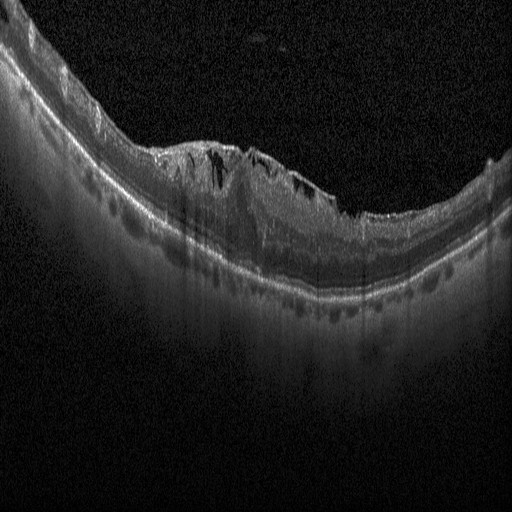 Macular OCT demonstrating diabetic macular edema.